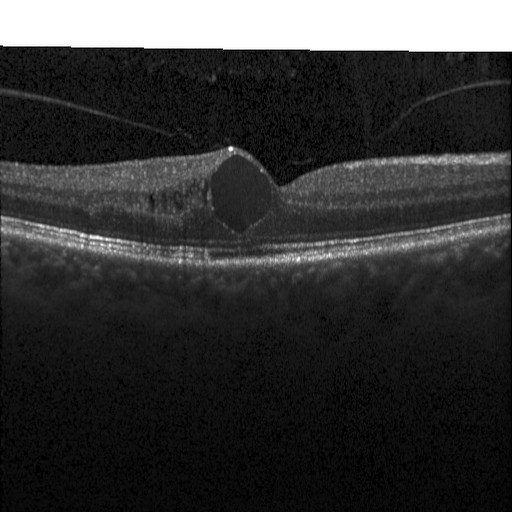

Diagnosis: diabetic macular edema.